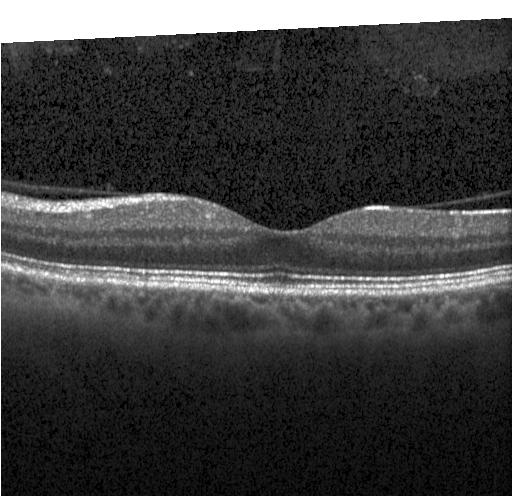

Horizontal scan through the fovea · OCT B-scan · Heidelberg Spectralis. OCT finding: no choroidal neovascularization, diabetic macular edema, or drusen.